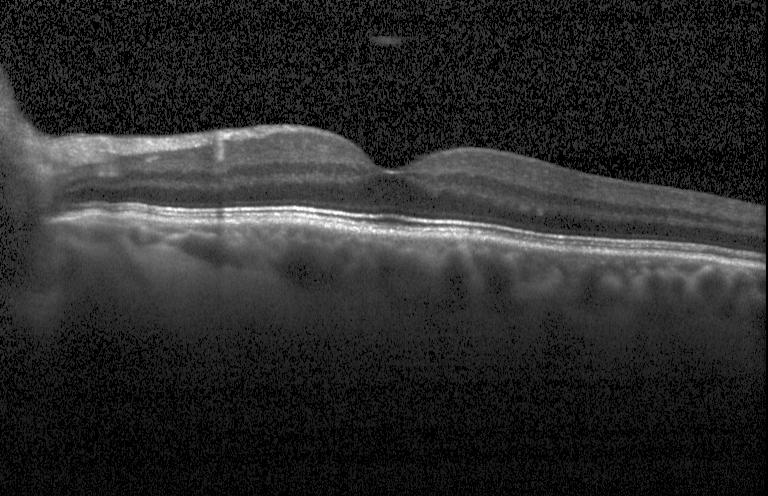 Finding: no evidence of CNV, DME, or drusen.